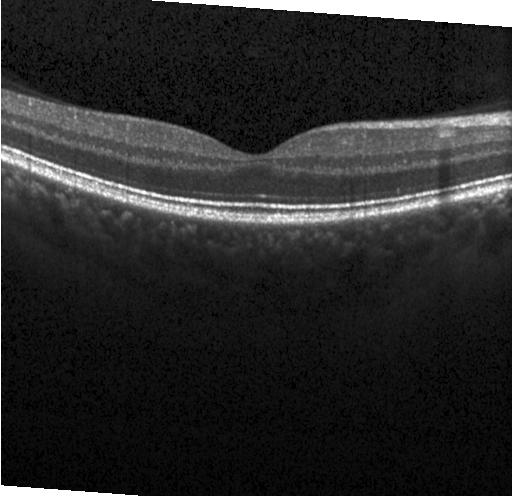 OCT B-scan.
Assessment: no choroidal neovascularization, diabetic macular edema, or drusen.